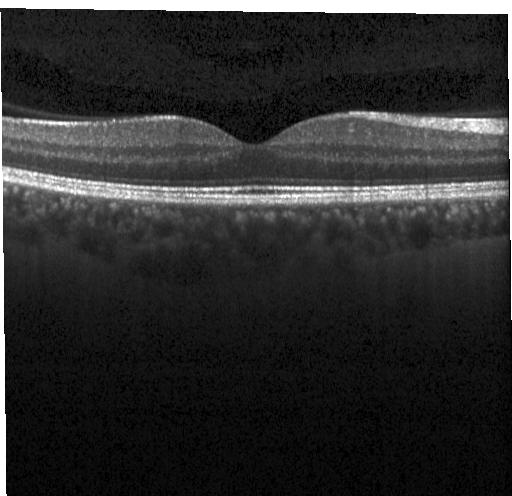
OCT B-scan showing no choroidal neovascularization, diabetic macular edema, or drusen.